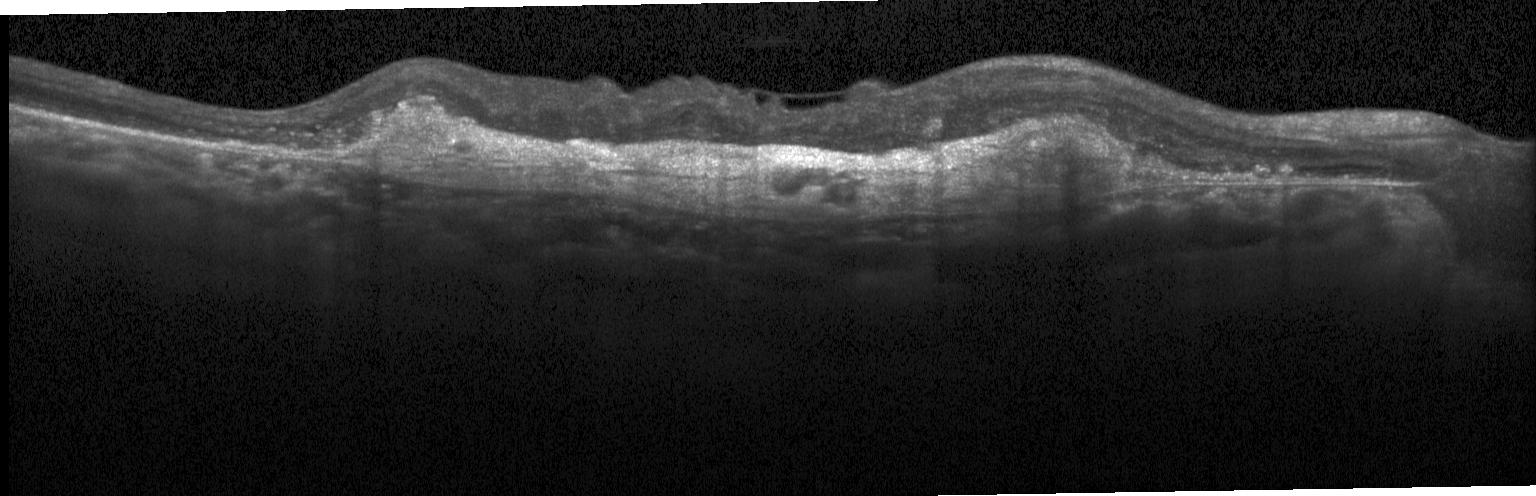

Impression: a choroidal neovascular membrane.